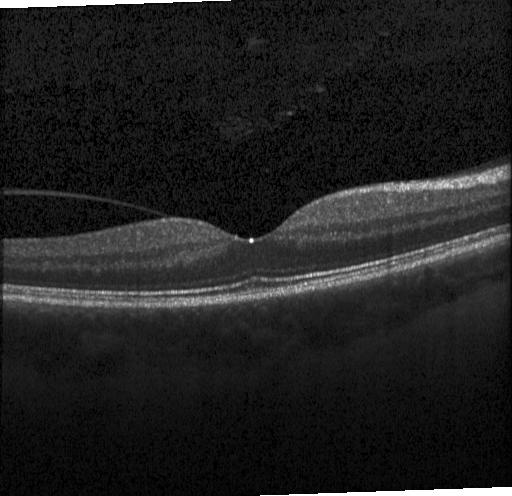
Macular scan; retinal OCT cross-section; spectral-domain OCT; acquired on a Heidelberg Spectralis. The scan shows neither choroidal neovascularization, diabetic macular edema, nor drusen.